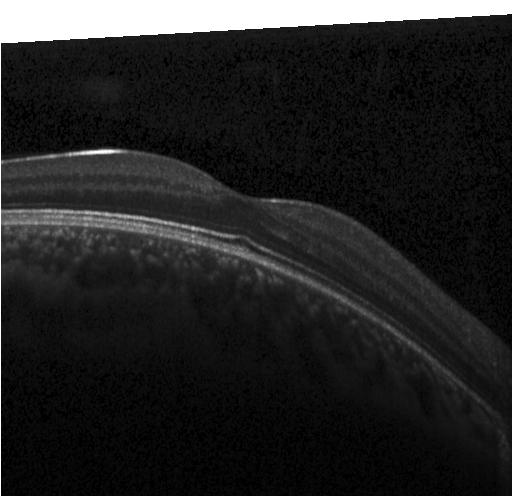

Impression: no choroidal neovascularization, no diabetic macular edema, and no drusen.